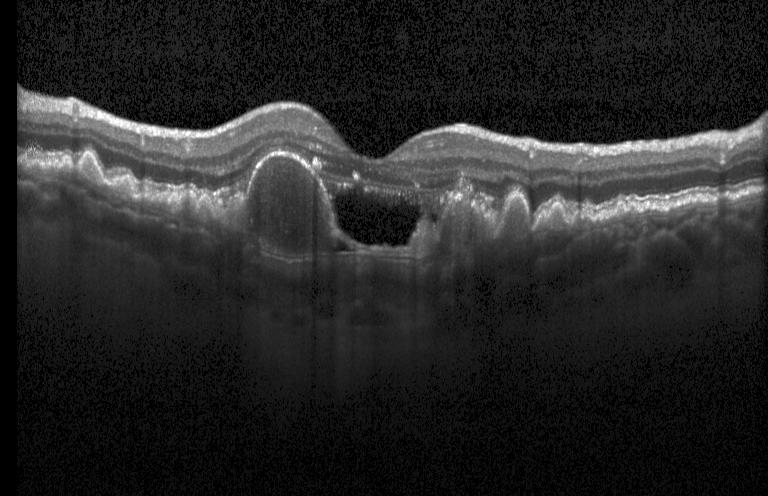
OCT line scan.
The scan shows a choroidal neovascular membrane.